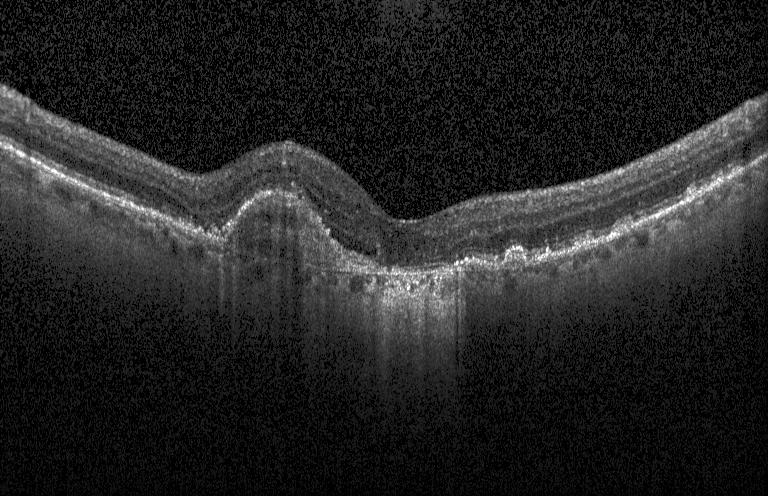
Optical coherence tomography B-scan. Spectral-domain optical coherence tomography. Macular scan. Heidelberg Spectralis. Impression: CNV.